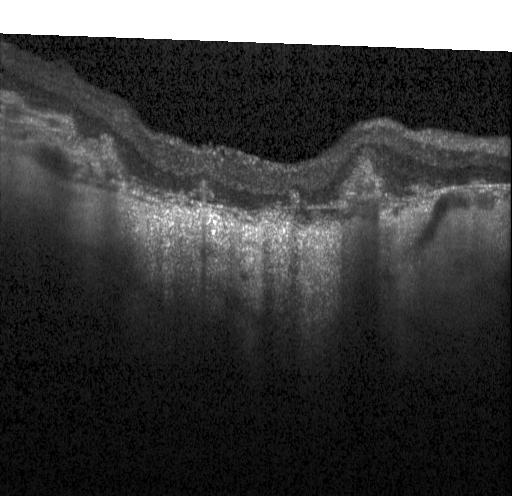

Macular OCT demonstrating a choroidal neovascular membrane.